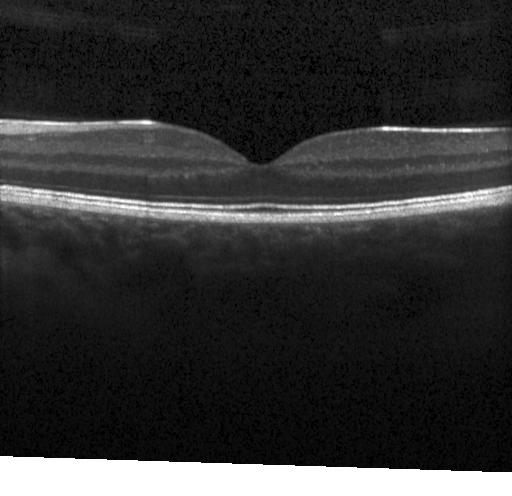
Spectral-domain OCT B-scan: no choroidal neovascularization, diabetic macular edema, or drusen.